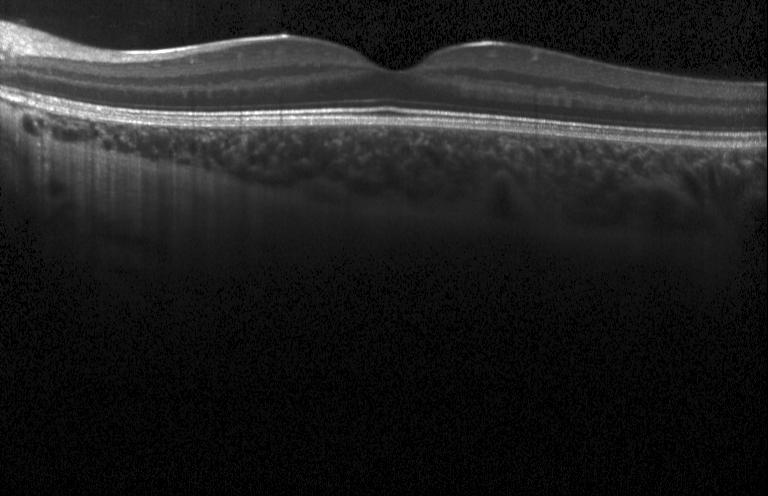

Through the macula. SD-OCT. Retinal OCT B-scan.
Finding: no choroidal neovascularization, no diabetic macular edema, and no drusen.